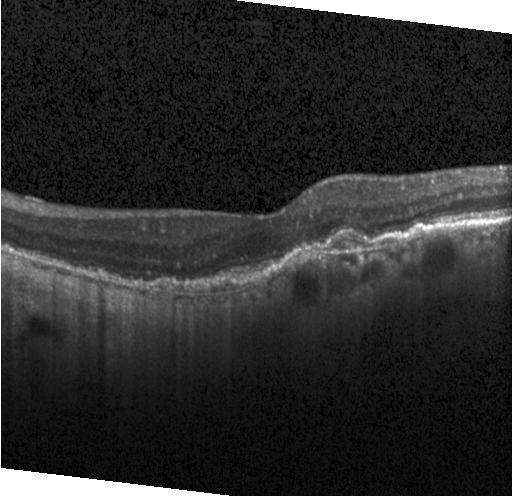 Optical coherence tomography scan. Finding: a choroidal neovascular membrane.